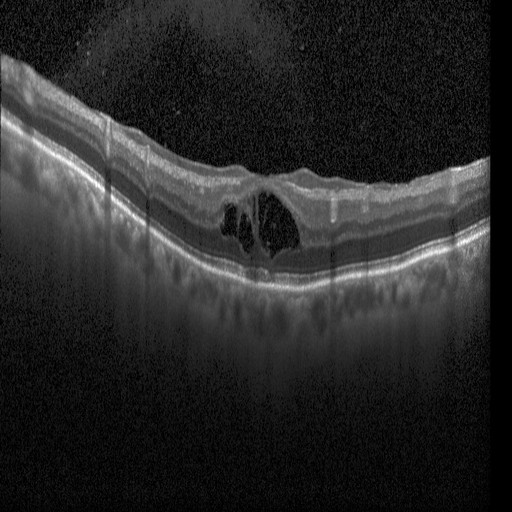

Retinal OCT B-scan
Macular OCT: DME.